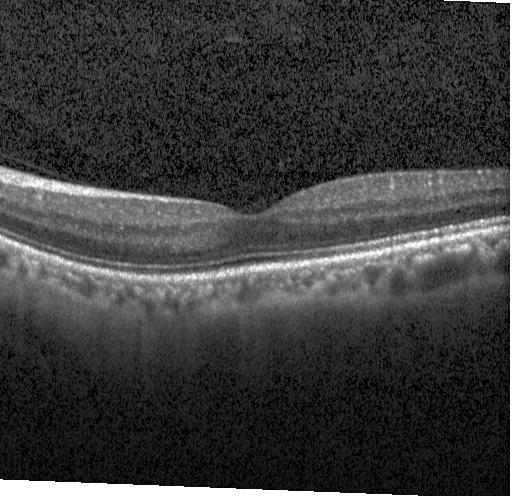

Macular OCT demonstrating neither CNV, DME, nor drusen.